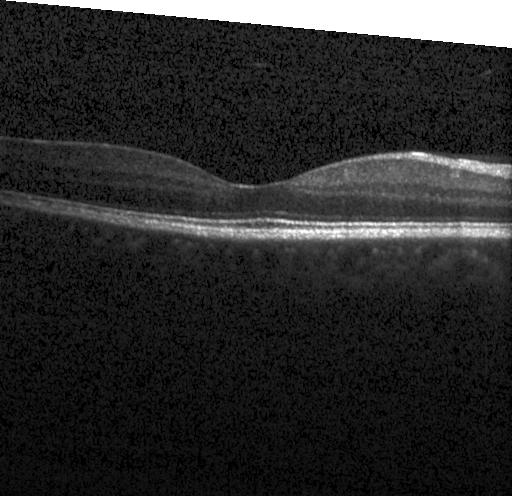

Optical coherence tomography B-scan; Heidelberg Spectralis; centered on the fovea; SD-OCT
No choroidal neovascularization, no diabetic macular edema, and no drusen.